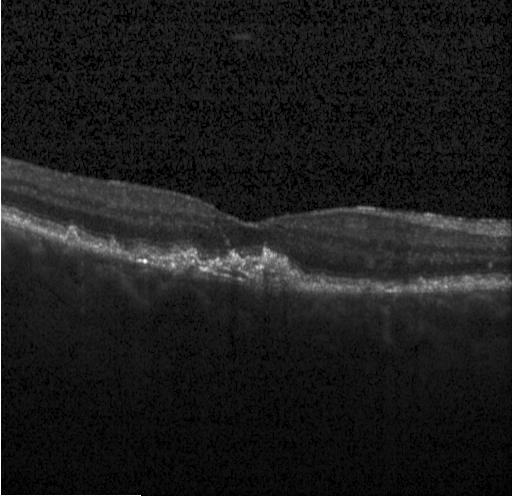

Retinal OCT B-scan.
This B-scan demonstrates a choroidal neovascular membrane.